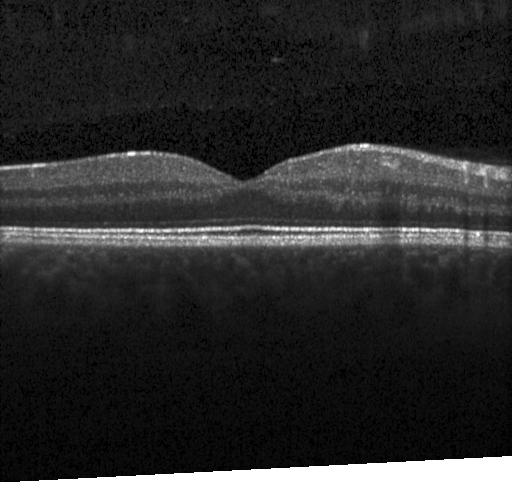
Heidelberg Spectralis, OCT line scan — Impression: no choroidal neovascularization, diabetic macular edema, or drusen.